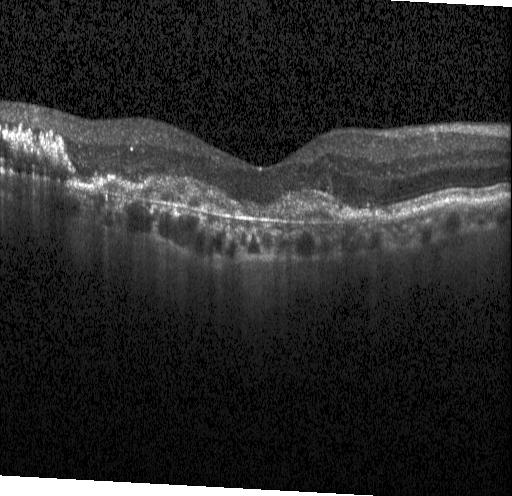
Heidelberg Spectralis OCT system; spectral-domain OCT; optical coherence tomography scan — Macular OCT: choroidal neovascularization.